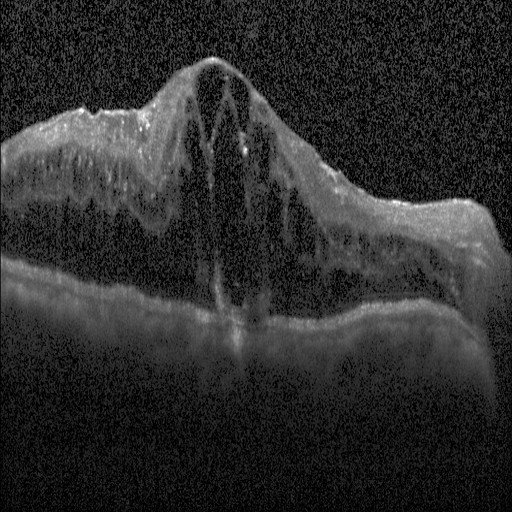 Diagnosis: DME.